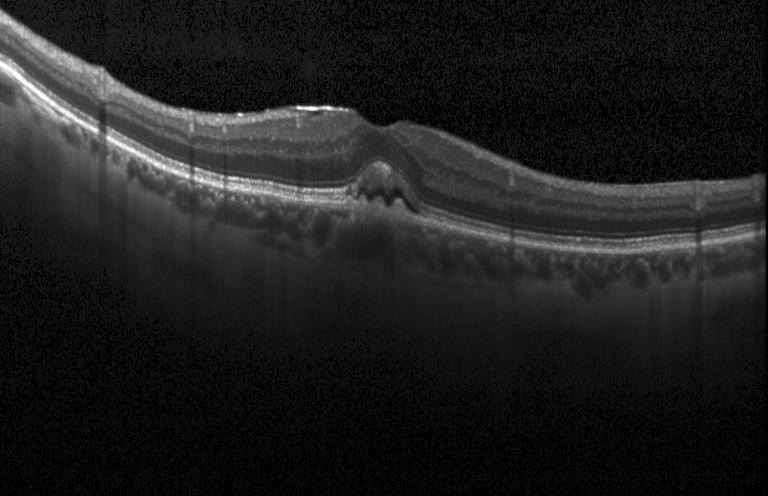 SD-OCT; OCT B-scan — Diagnosis: a choroidal neovascular membrane.